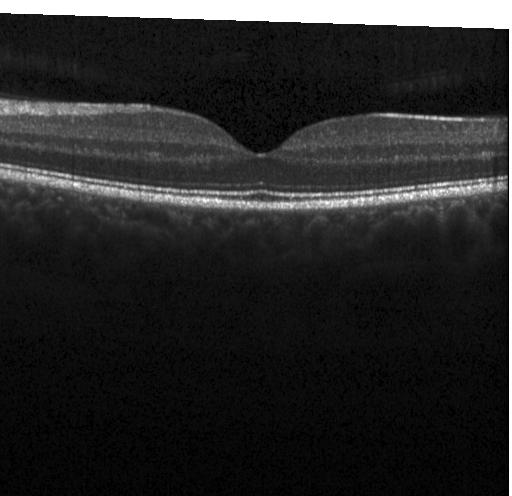
Heidelberg Spectralis OCT system · retinal OCT B-scan. Assessment: neither choroidal neovascularization, diabetic macular edema, nor drusen.